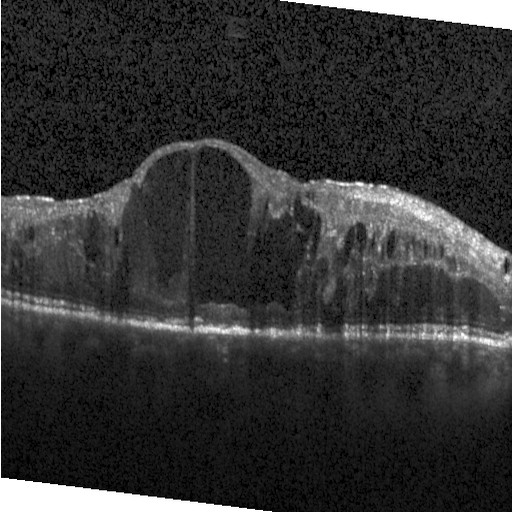
OCT line scan.
Impression: DME.